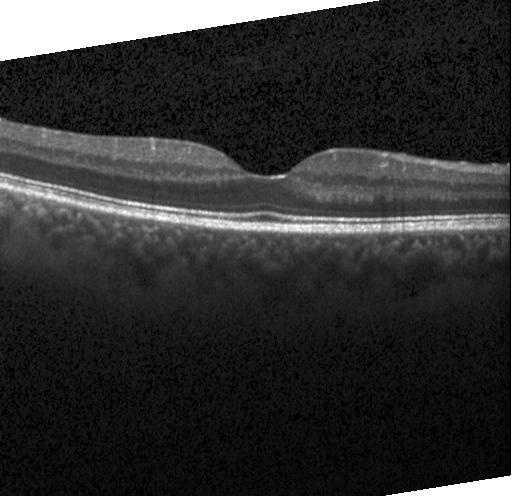 Retinal OCT B-scan, spectral-domain OCT, macular scan.
Diagnosis: no CNV, no DME, and no drusen.